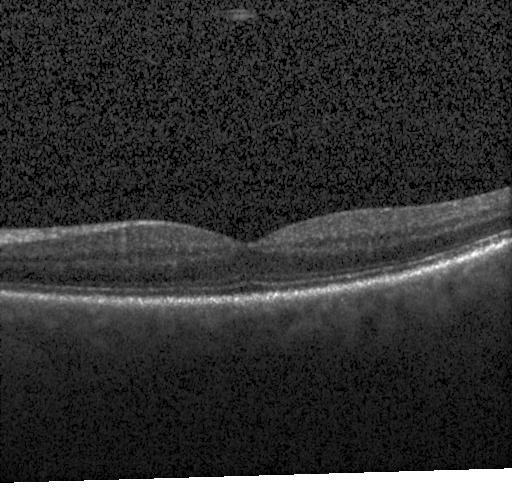

Spectral-domain OCT B-scan: no CNV, no DME, and no drusen.